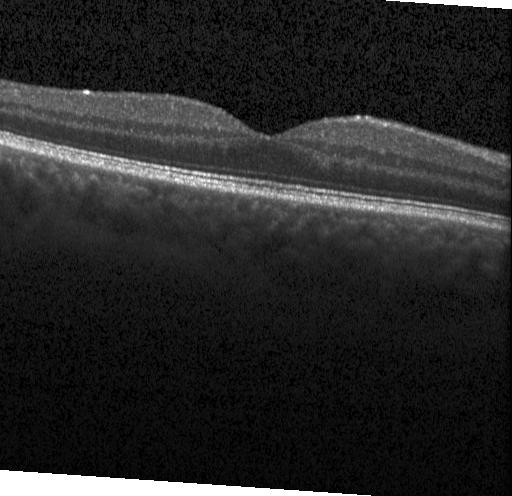 Finding: no evidence of choroidal neovascularization, diabetic macular edema, or drusen.